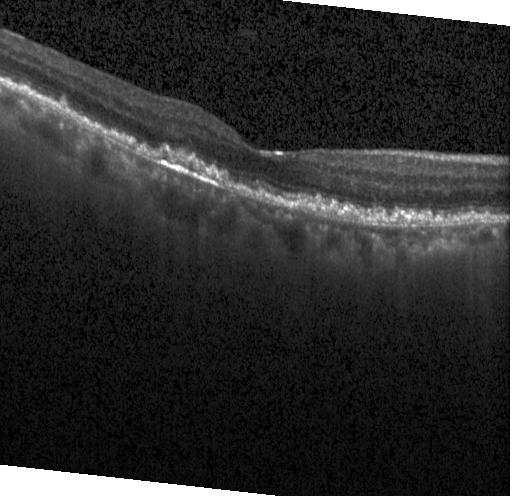

SD-OCT; Heidelberg Spectralis; OCT B-scan. This B-scan demonstrates drusen.